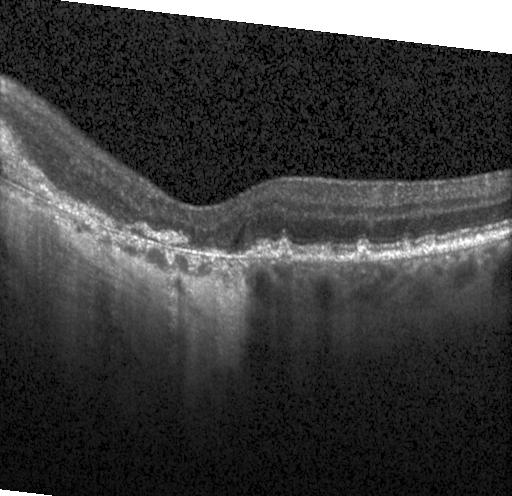

OCT B-scan. The scan shows choroidal neovascularization.